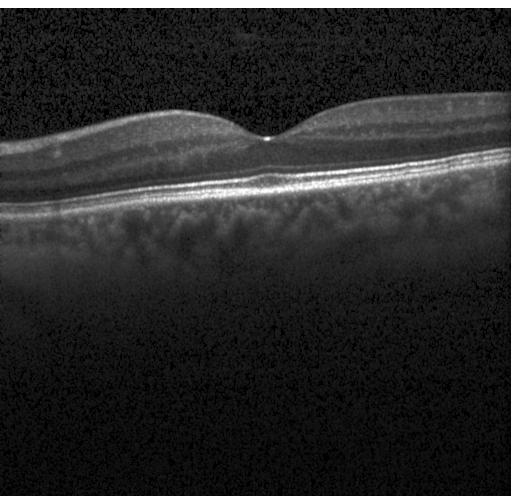

Optical coherence tomography scan. Fovea-centered. Instrument: Heidelberg Spectralis. Spectral-domain OCT. Assessment: no CNV, no DME, and no drusen.